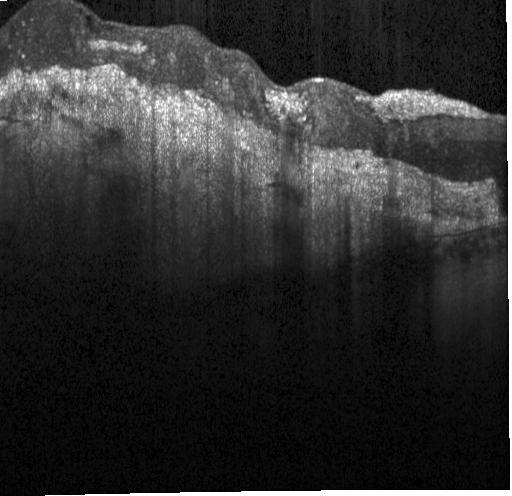
Diagnosis: a choroidal neovascular membrane.